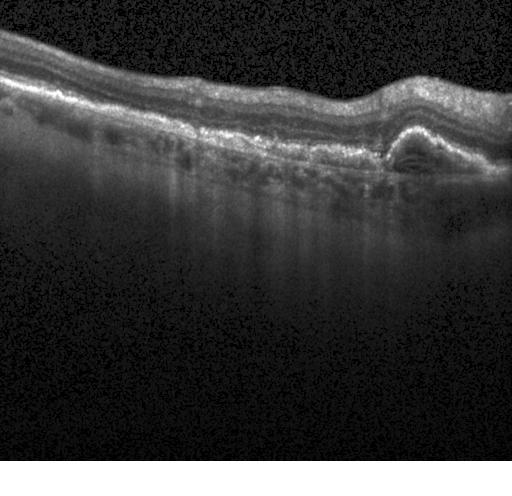 Optical coherence tomography scan · SD-OCT · acquired on a Heidelberg Spectralis
OCT finding: a choroidal neovascular membrane.